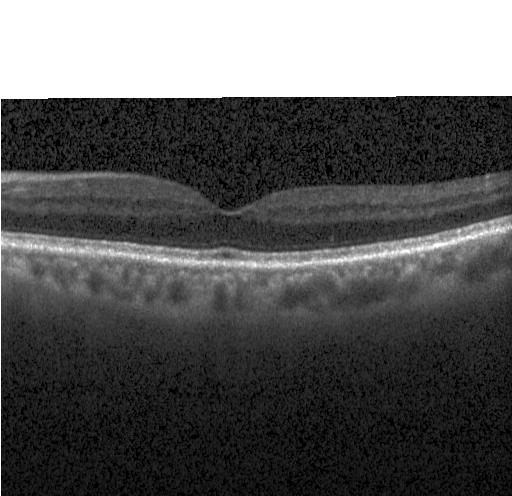

Retinal OCT cross-section — Dx: no evidence of choroidal neovascularization, diabetic macular edema, or drusen.